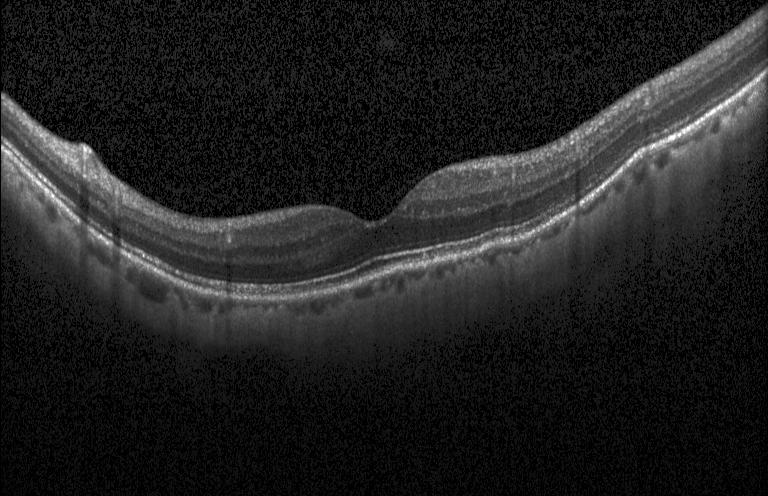
Acquired on a Heidelberg Spectralis; OCT line scan. The scan shows neither CNV, DME, nor drusen.